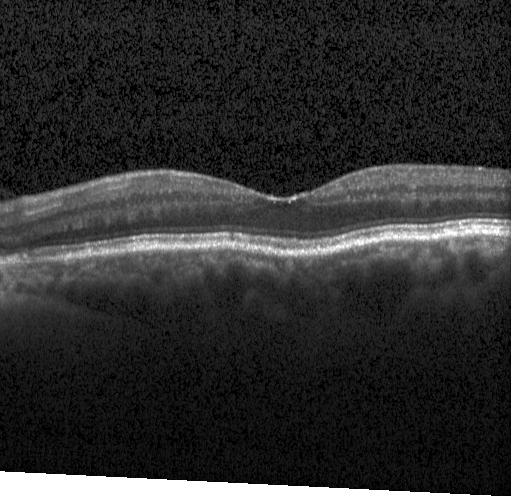
Horizontal scan through the fovea. Optical coherence tomography scan
Diagnosis: no choroidal neovascularization, diabetic macular edema, or drusen.